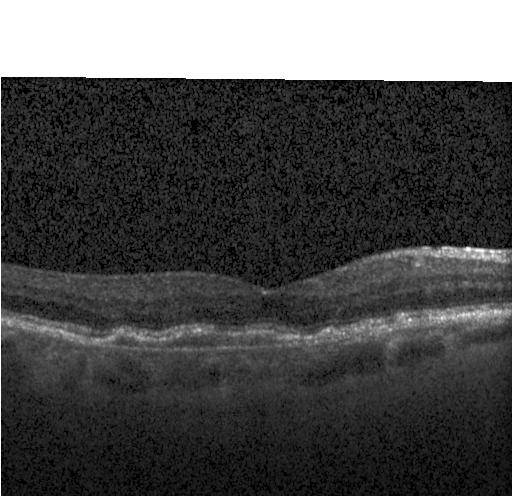
Retinal OCT cross-section, through the macula, spectral-domain optical coherence tomography
The scan shows a choroidal neovascular membrane.